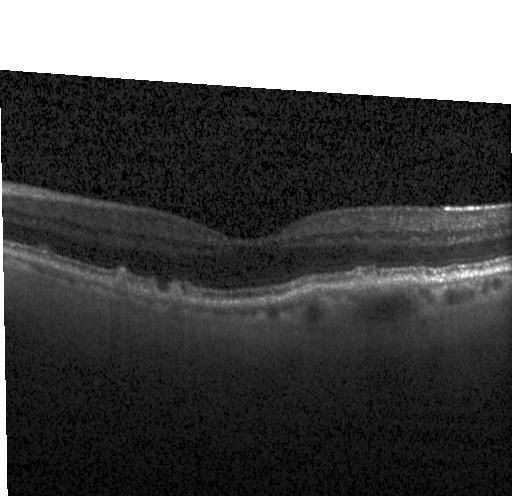 OCT B-scan, macular scan, instrument: Heidelberg Spectralis.
Impression: multiple drusen.